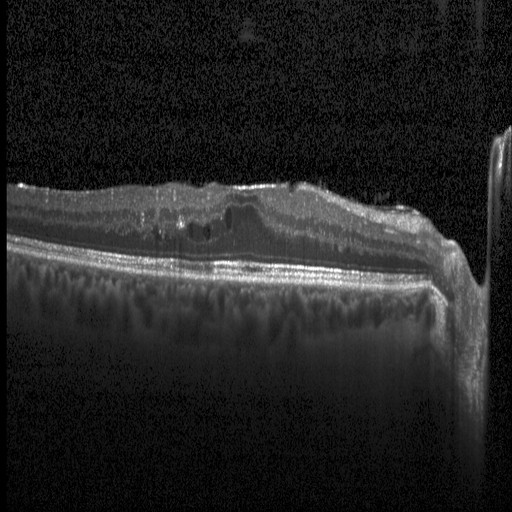 Optical coherence tomography scan
Diabetic macular edema.